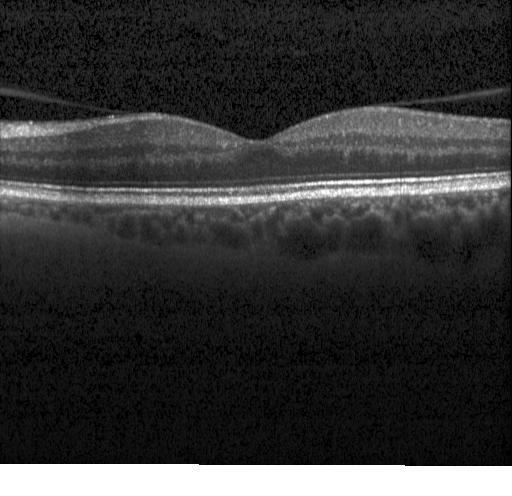 Through the macula; instrument: Heidelberg Spectralis; spectral-domain optical coherence tomography; optical coherence tomography B-scan
Diagnosis: no choroidal neovascularization, no diabetic macular edema, and no drusen.